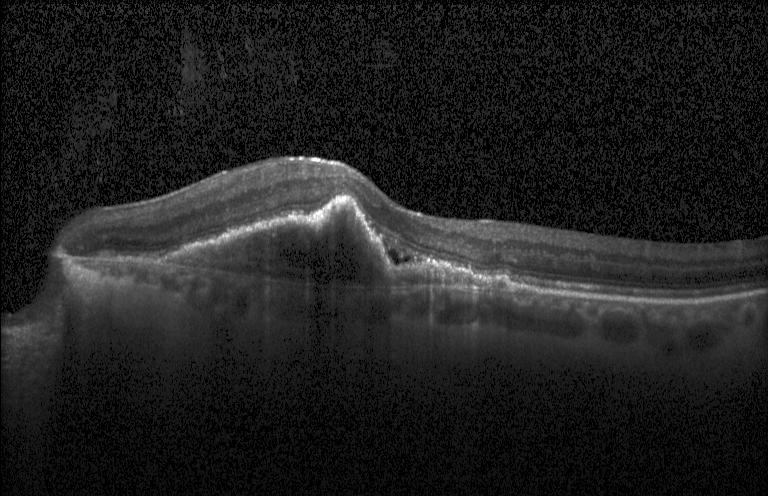 Fovea-centered, Heidelberg Spectralis OCT system, retinal OCT cross-section, spectral-domain optical coherence tomography.
Assessment: CNV.